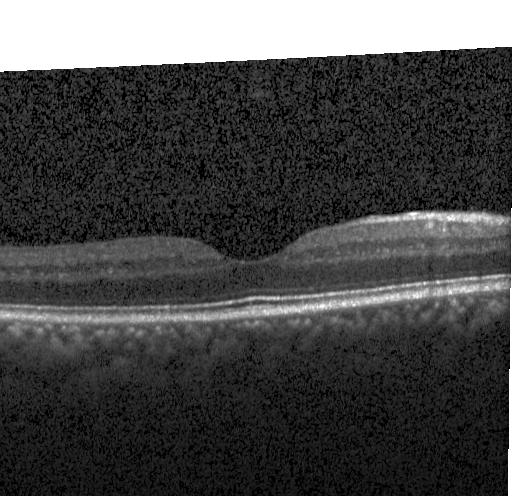
Fovea-centered; instrument: Heidelberg Spectralis; spectral-domain optical coherence tomography; optical coherence tomography scan.
Assessment: no choroidal neovascularization, no diabetic macular edema, and no drusen.